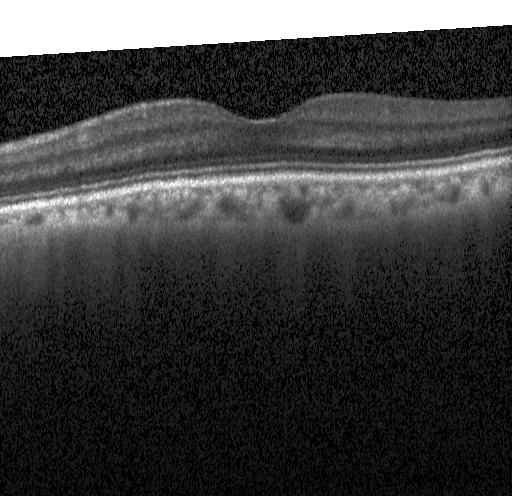

Impression: no evidence of choroidal neovascularization, diabetic macular edema, or drusen.